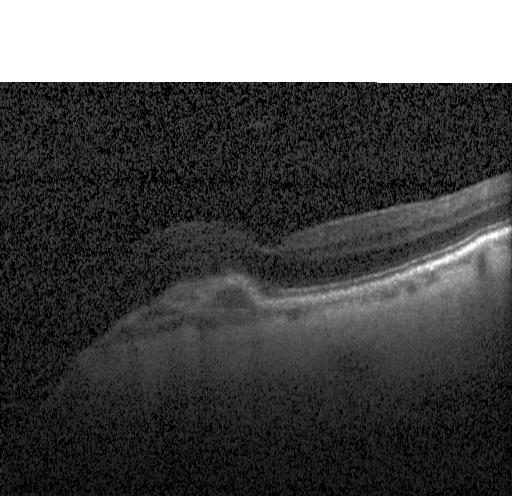 Dx: a choroidal neovascular membrane.